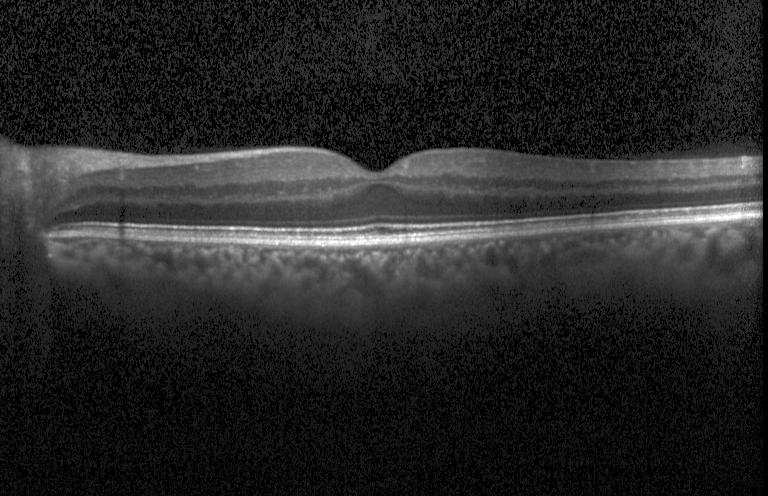 Heidelberg Spectralis OCT system. SD-OCT. Horizontal scan through the fovea. Optical coherence tomography B-scan — Assessment: neither CNV, DME, nor drusen.